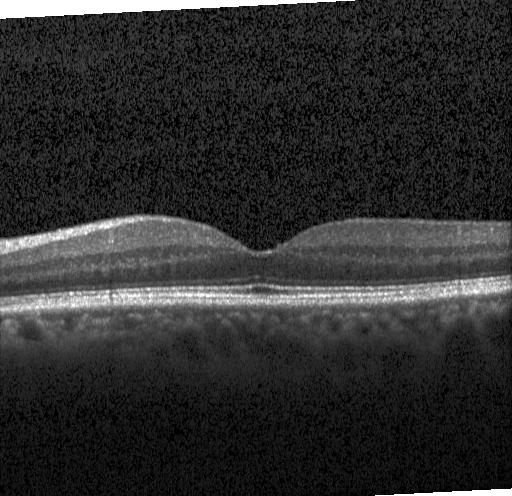
Spectral-domain OCT · OCT line scan · centered on the fovea — OCT finding: no CNV, DME, or drusen.